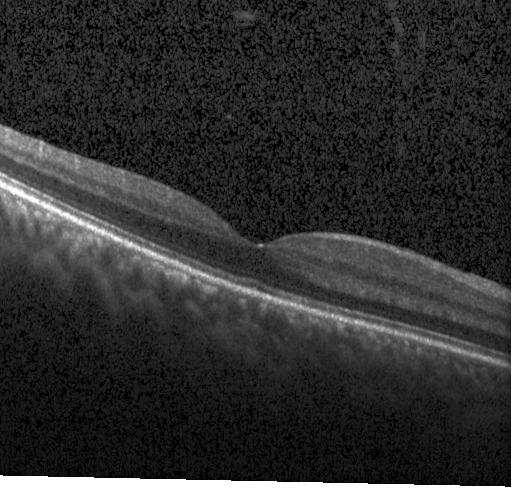

OCT B-scan showing no CNV, no DME, and no drusen.